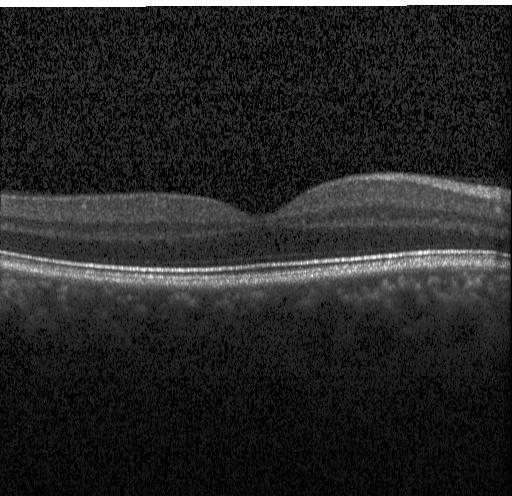 This B-scan demonstrates no choroidal neovascularization, diabetic macular edema, or drusen.